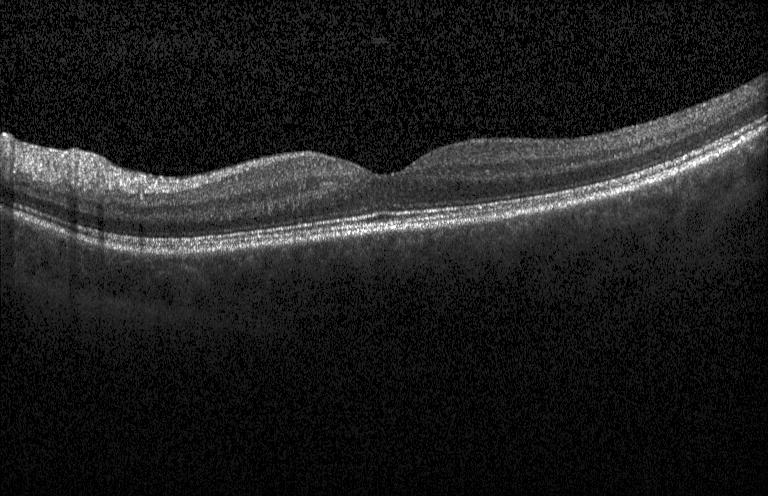
OCT line scan, acquired on a Heidelberg Spectralis, through the macula, spectral-domain OCT — Impression: no evidence of CNV, DME, or drusen.